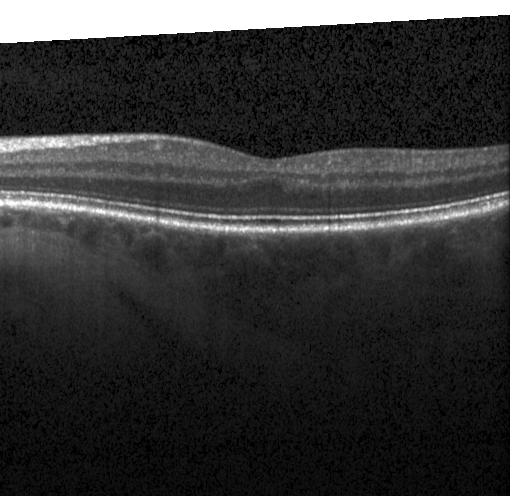 Macular OCT: neither choroidal neovascularization, diabetic macular edema, nor drusen.